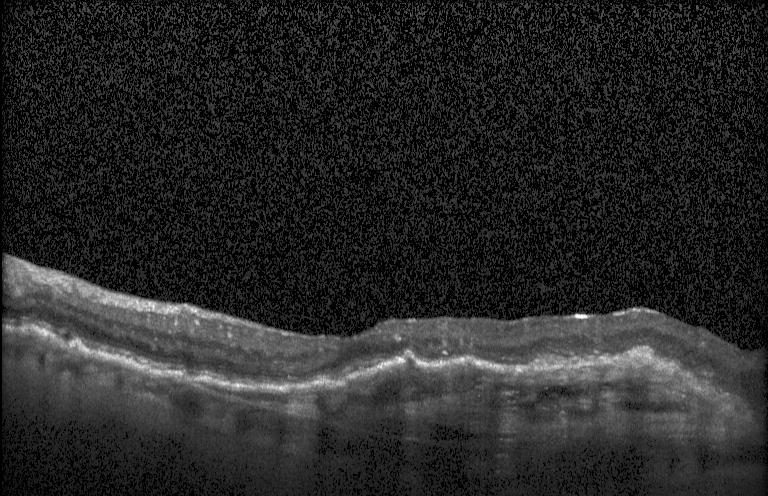
OCT scan showing a choroidal neovascular membrane.